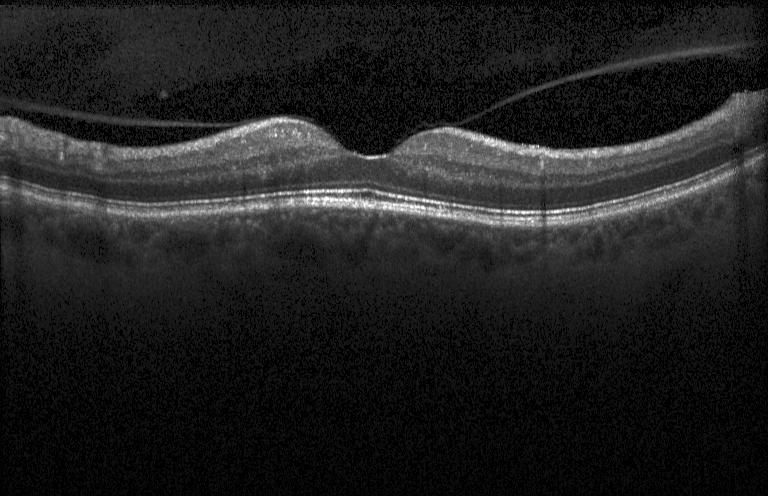
Diagnosis: no choroidal neovascularization, diabetic macular edema, or drusen.